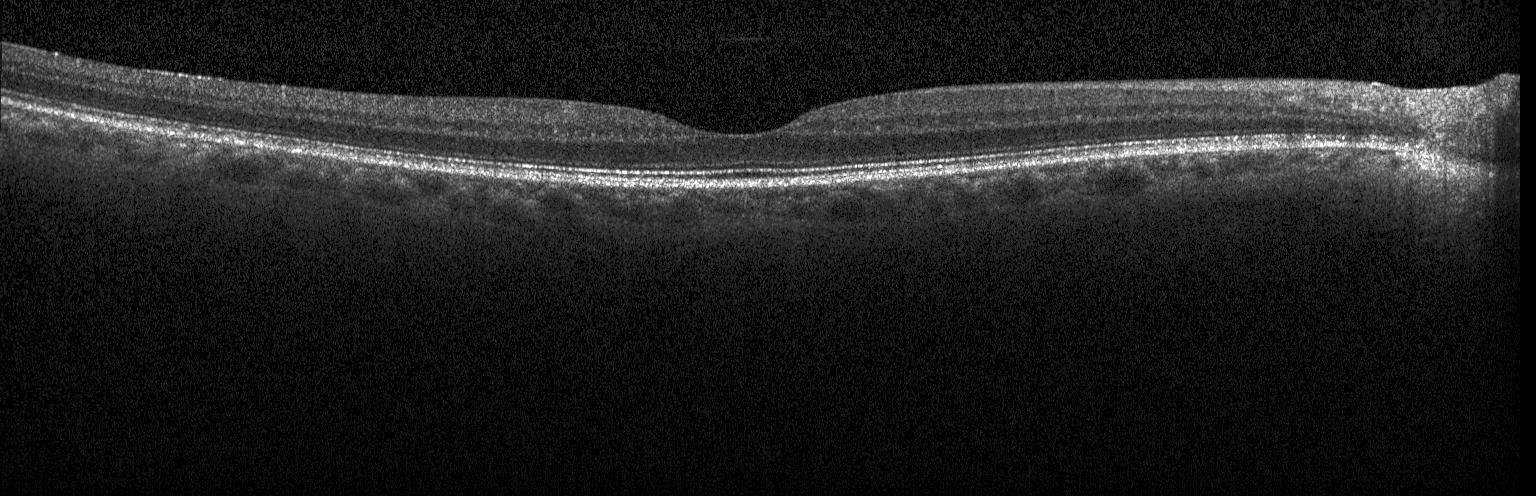 OCT finding: no evidence of choroidal neovascularization, diabetic macular edema, or drusen.